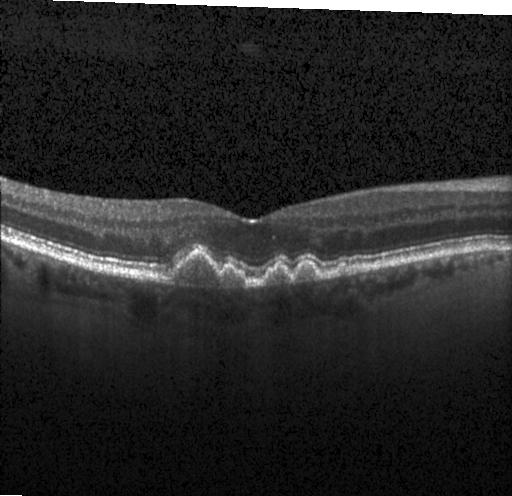
Macular scan. OCT B-scan.
Finding: drusen.